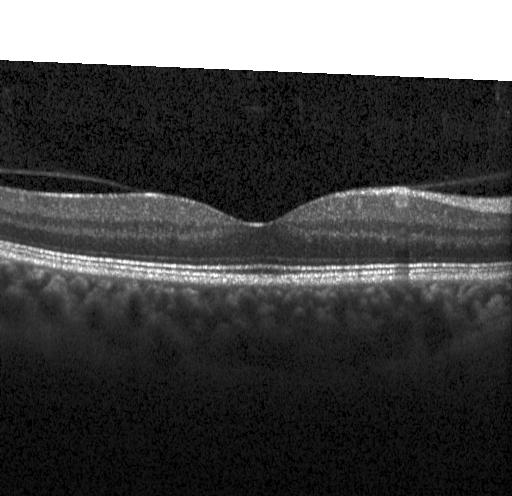
Centered on the fovea; Heidelberg Spectralis; optical coherence tomography scan; SD-OCT — Finding: no CNV, no DME, and no drusen.